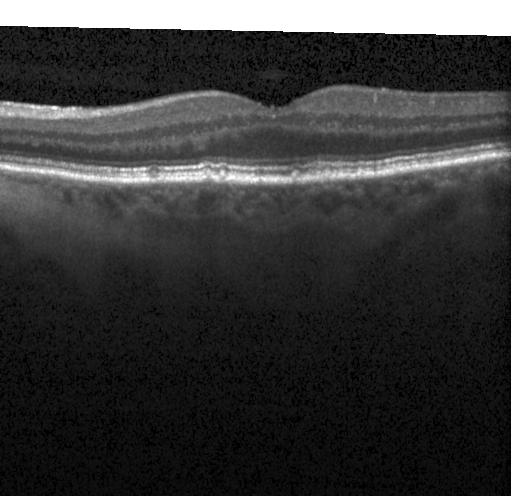 OCT scan showing drusen.